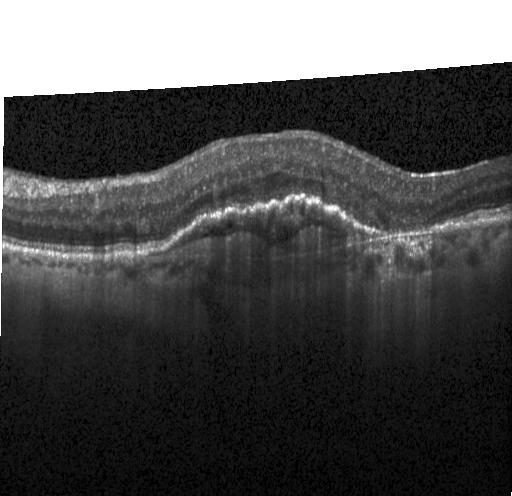
Acquired on a Heidelberg Spectralis · optical coherence tomography B-scan — OCT finding: a choroidal neovascular membrane.